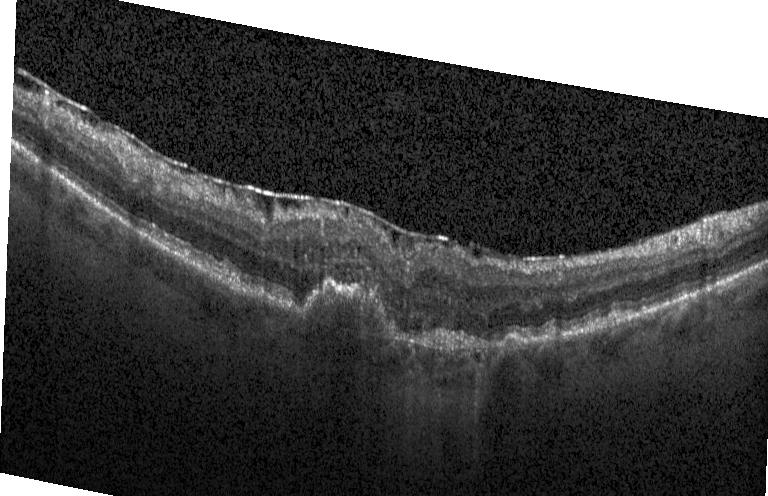
Retinal OCT B-scan. Assessment: choroidal neovascularization (CNV).